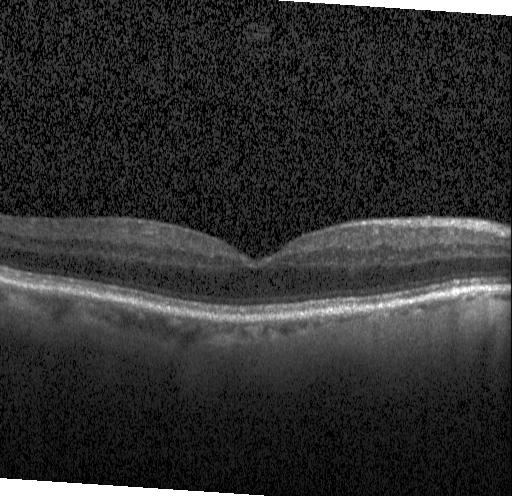

Centered on the fovea, instrument: Heidelberg Spectralis, retinal OCT cross-section, spectral-domain OCT — Diagnosis: no choroidal neovascularization, no diabetic macular edema, and no drusen.